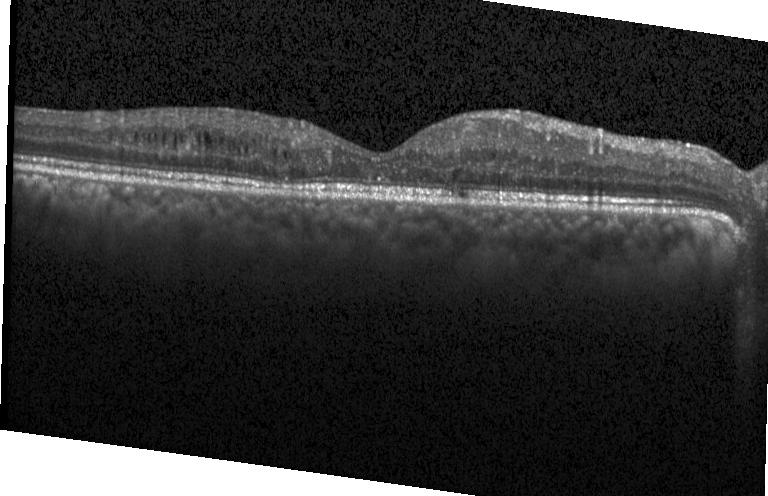

Diagnosis: diabetic macular edema (DME).